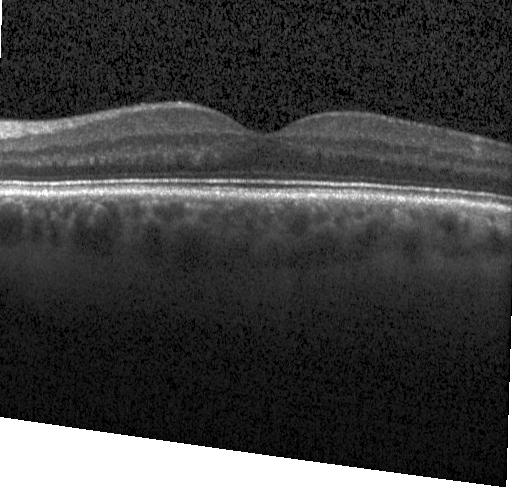
Retinal OCT B-scan. Centered on the fovea.
Diagnosis: neither choroidal neovascularization, diabetic macular edema, nor drusen.